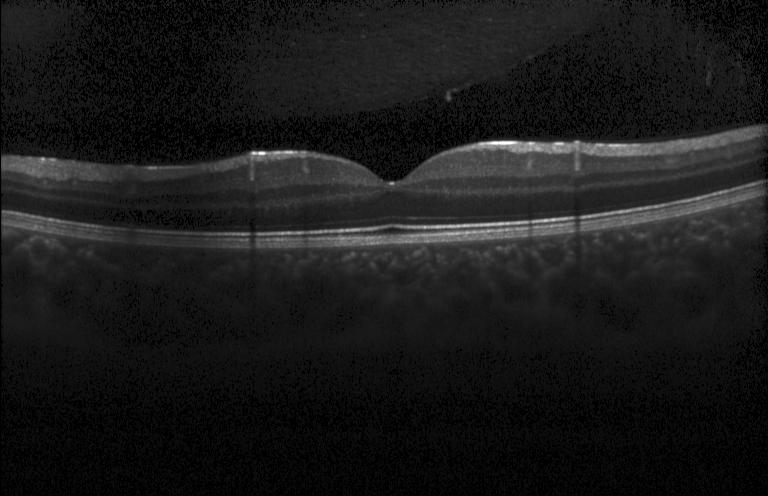

Optical coherence tomography scan; SD-OCT.
Finding: neither choroidal neovascularization, diabetic macular edema, nor drusen.